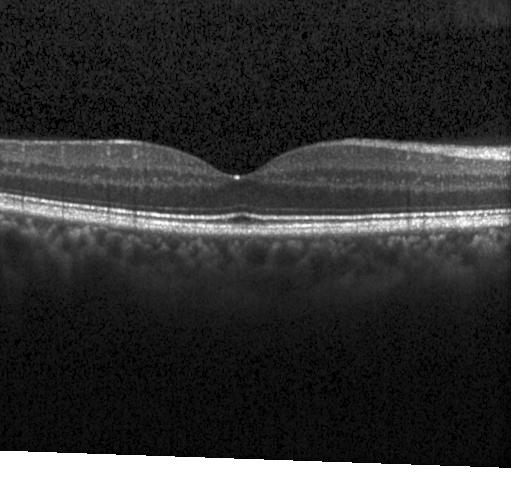
OCT B-scan showing no choroidal neovascularization, no diabetic macular edema, and no drusen.